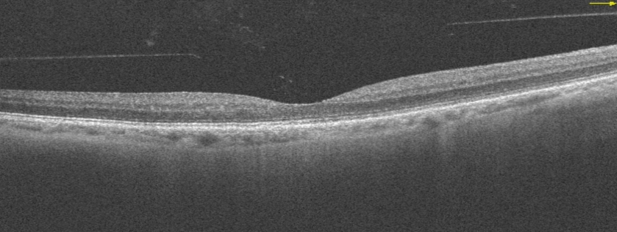 Impression: no AMD, DME, ERM, RAO, RVO, or VID.